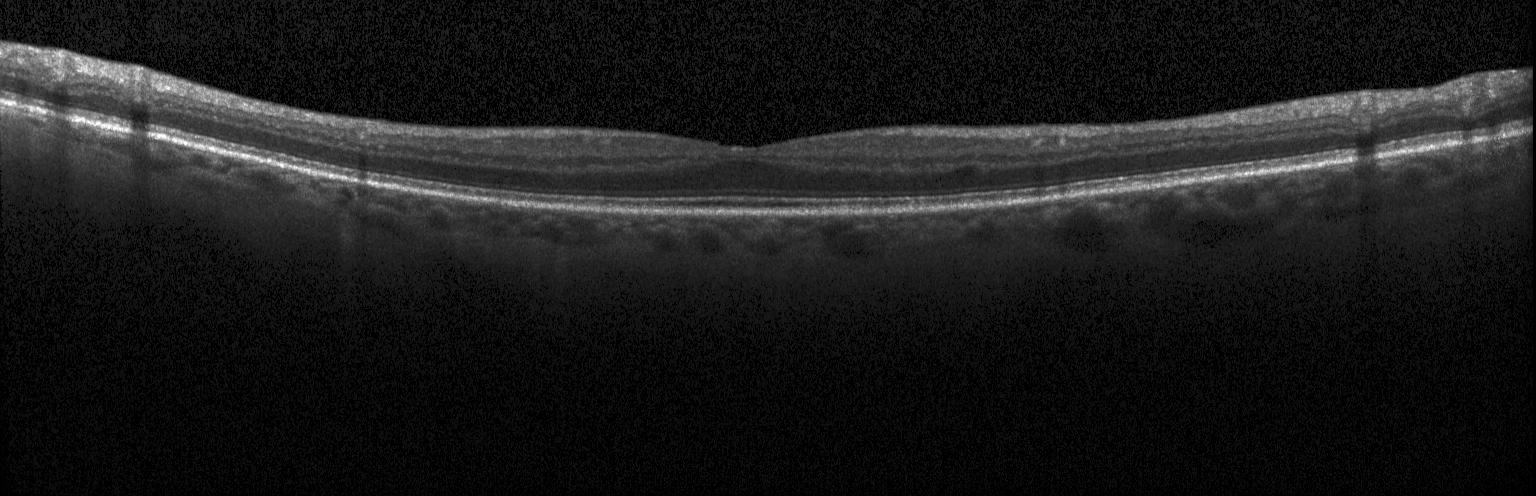

Instrument: Heidelberg Spectralis; SD-OCT; OCT line scan
No choroidal neovascularization, diabetic macular edema, or drusen.